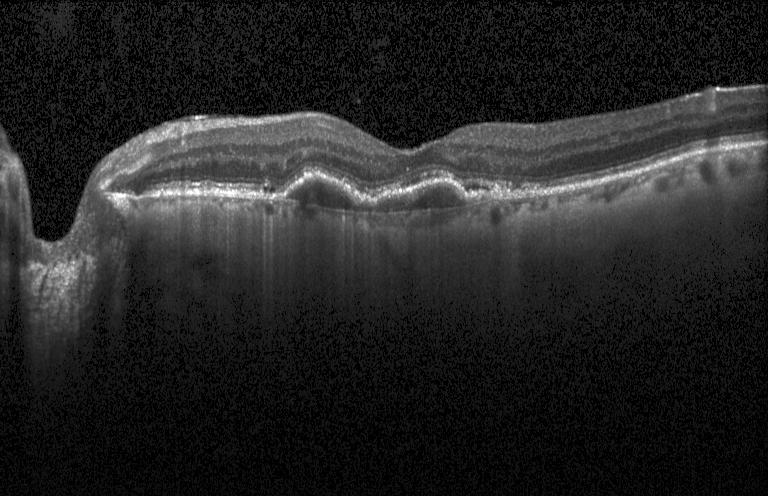 Spectral-domain OCT. OCT B-scan — A choroidal neovascular membrane.